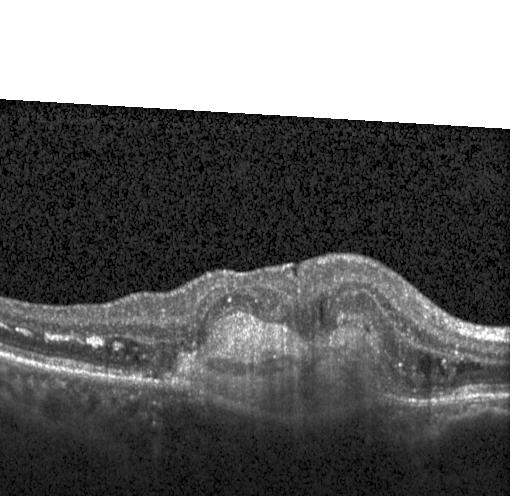 Diagnosis: choroidal neovascularization (CNV).